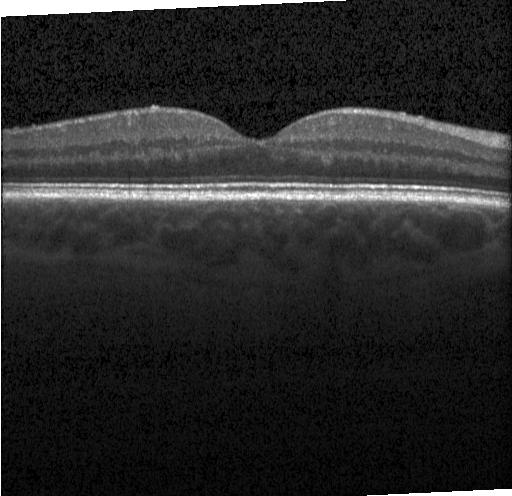
Impression: no CNV, DME, or drusen.